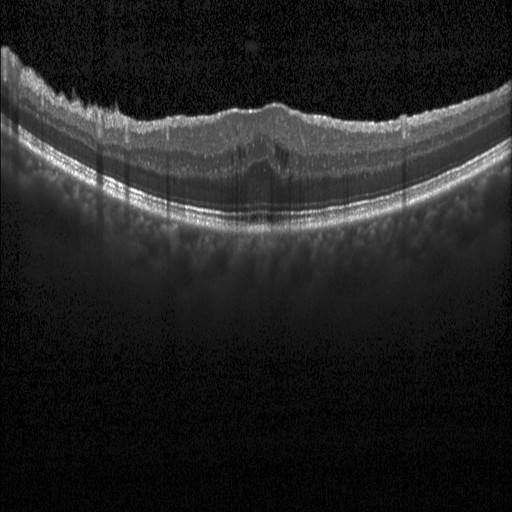
Optical coherence tomography B-scan — The scan shows diabetic macular edema (DME).